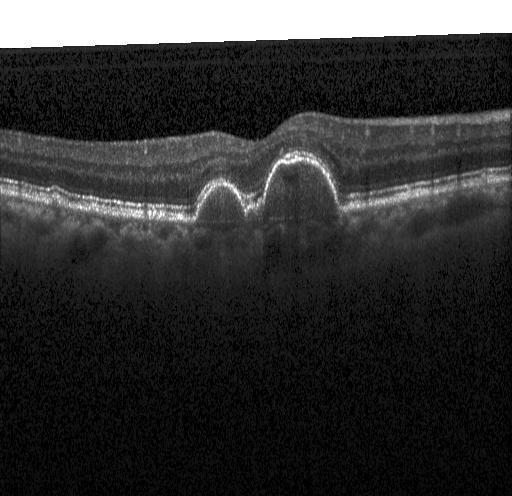 Spectral-domain OCT B-scan: sub-RPE drusenoid deposits.